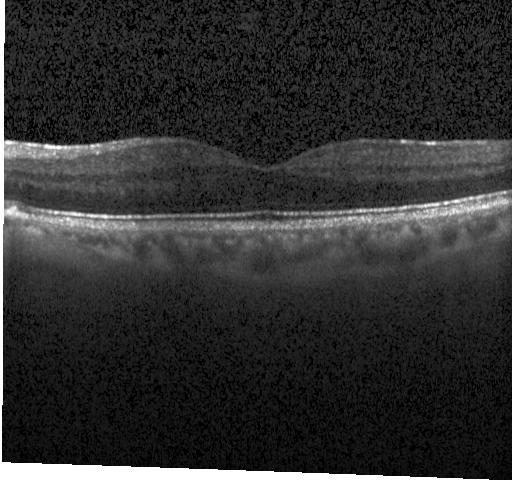 Spectral-domain OCT; Heidelberg Spectralis; retinal OCT B-scan.
Diagnosis: no CNV, DME, or drusen.